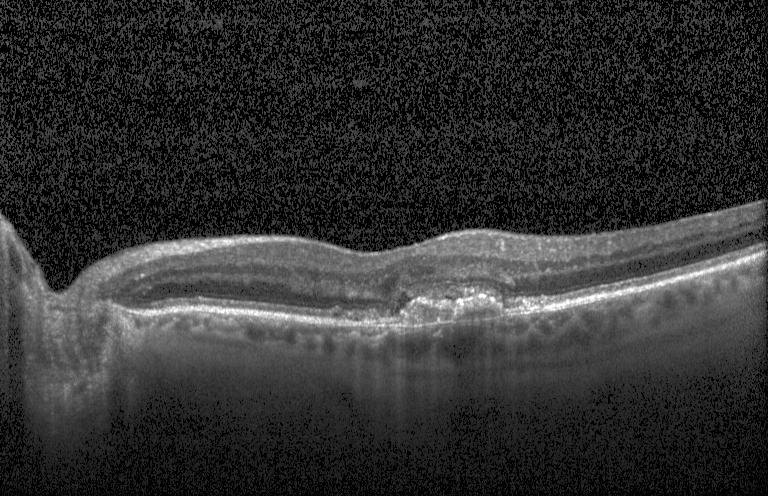

OCT line scan, fovea-centered — Finding: a choroidal neovascular membrane.